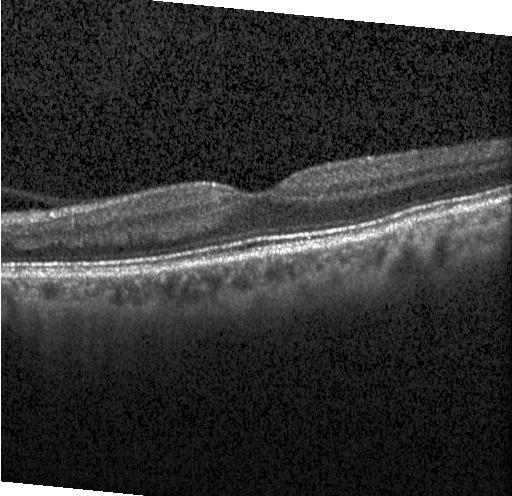

Spectral-domain OCT. Horizontal scan through the fovea. OCT line scan
No evidence of choroidal neovascularization, diabetic macular edema, or drusen.